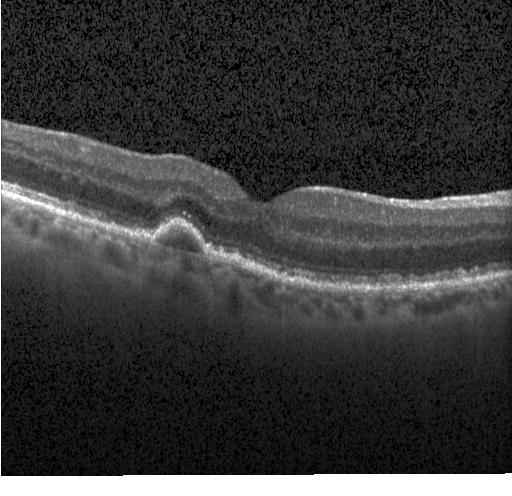
Horizontal scan through the fovea · retinal OCT B-scan · instrument: Heidelberg Spectralis · spectral-domain OCT.
Finding: multiple drusen.